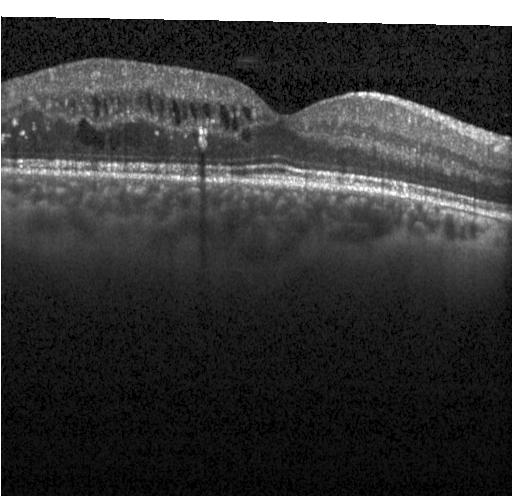
Diagnosis: diabetic macular edema (DME).